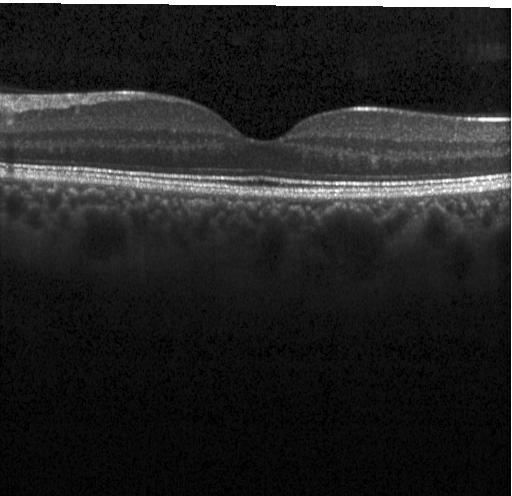 Fovea-centered · spectral-domain OCT · retinal OCT cross-section.
Macular OCT: neither choroidal neovascularization, diabetic macular edema, nor drusen.